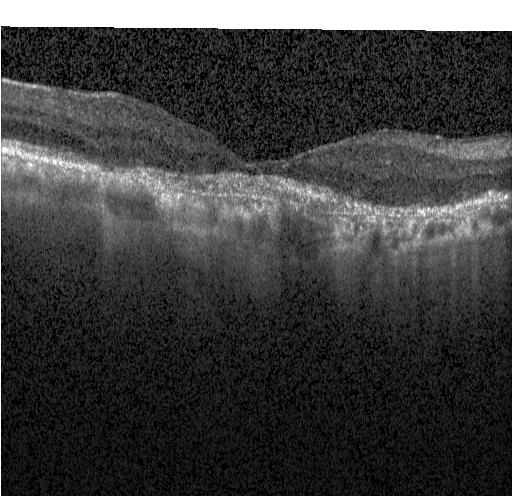
OCT line scan · spectral-domain OCT
The scan shows a choroidal neovascular membrane.